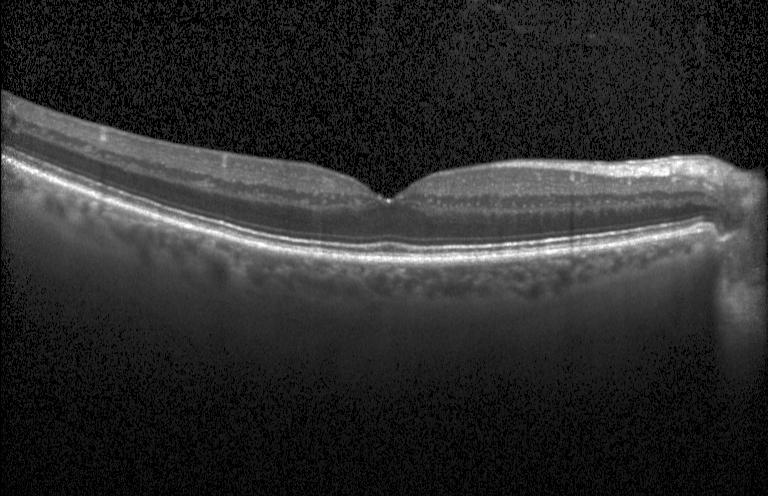

OCT line scan
Macular OCT: no CNV, DME, or drusen.